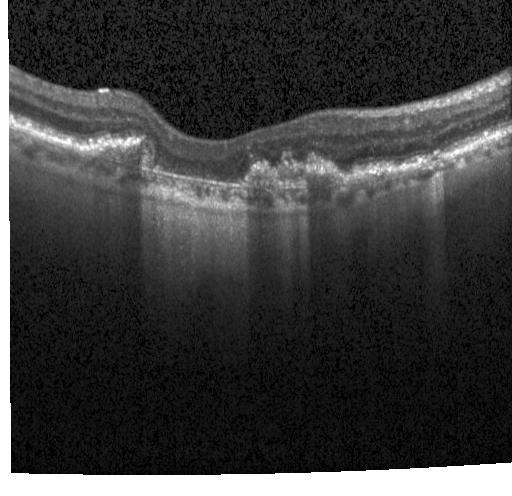

OCT line scan, instrument: Heidelberg Spectralis, centered on the fovea.
The scan shows CNV.